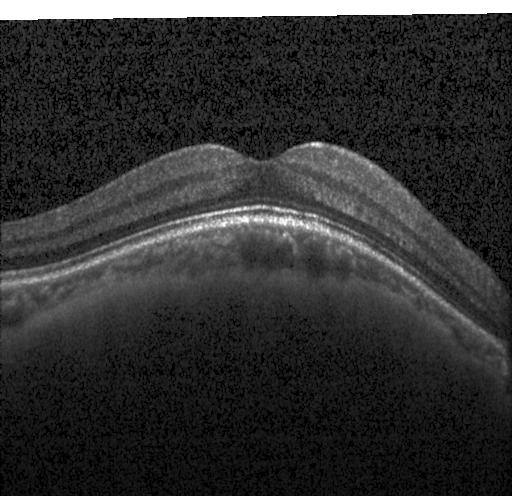
Macular scan. Instrument: Heidelberg Spectralis. Spectral-domain OCT. Optical coherence tomography scan.
Macular OCT: no evidence of choroidal neovascularization, diabetic macular edema, or drusen.